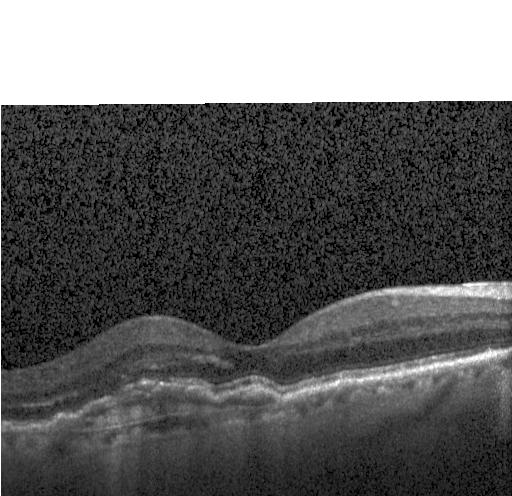 OCT B-scan. OCT finding: CNV.